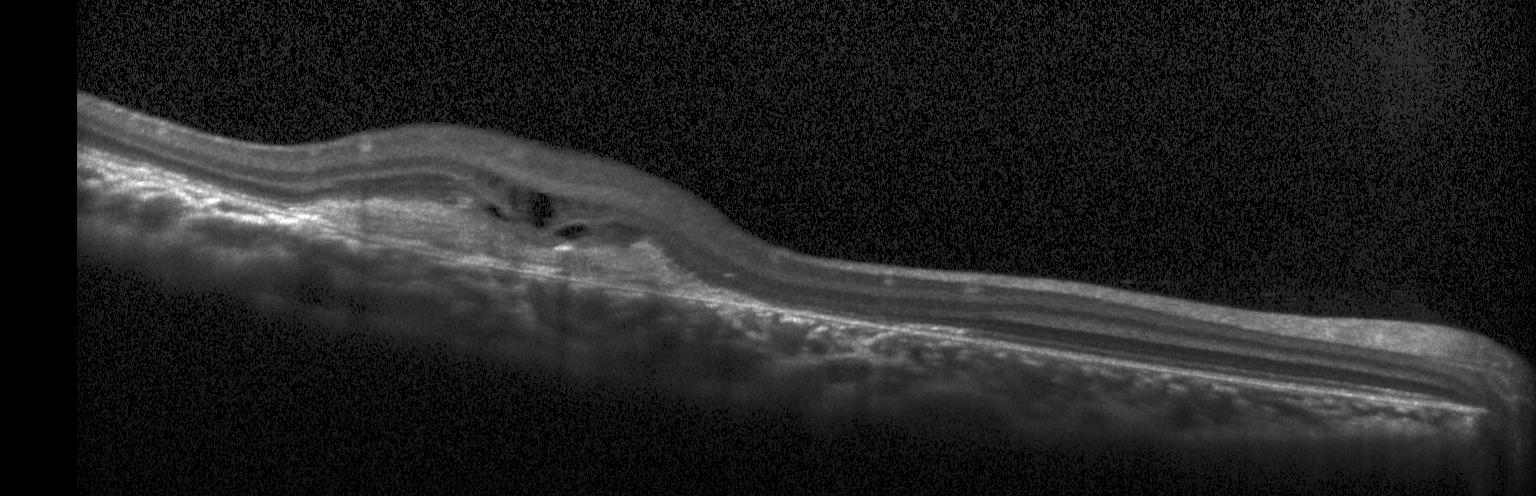

Through the macula. Retinal OCT B-scan. Spectral-domain optical coherence tomography. Instrument: Heidelberg Spectralis.
Assessment: a choroidal neovascular membrane.